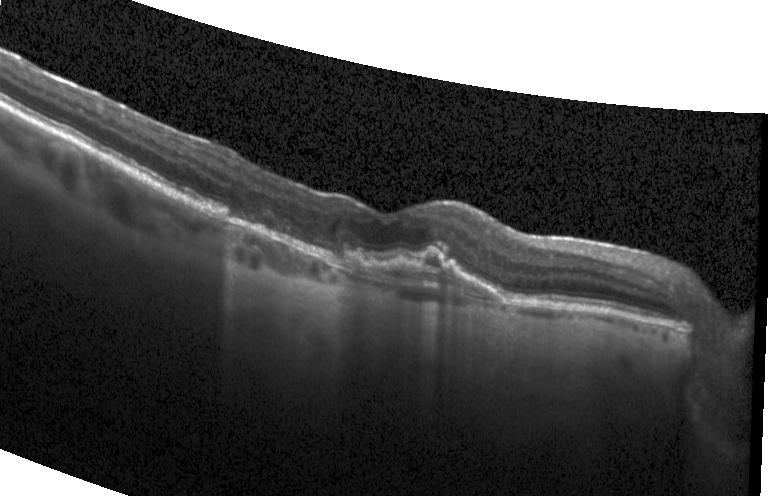
Finding: a choroidal neovascular membrane.